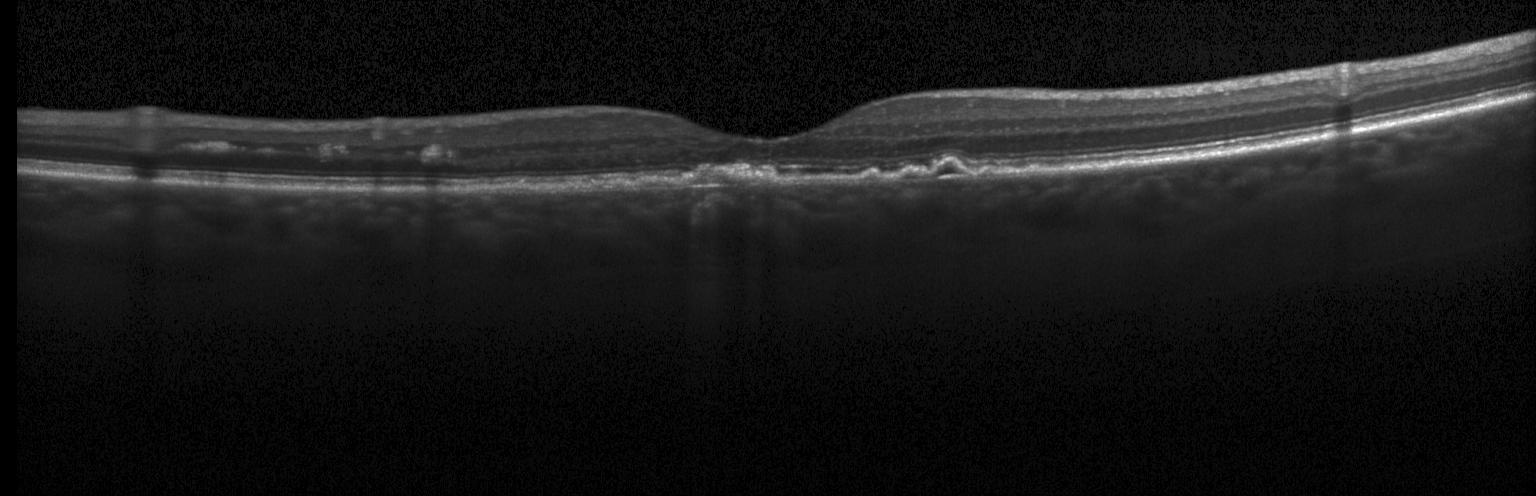

Retinal OCT B-scan · Heidelberg Spectralis OCT system · spectral-domain optical coherence tomography · through the macula. OCT finding: a choroidal neovascular membrane.